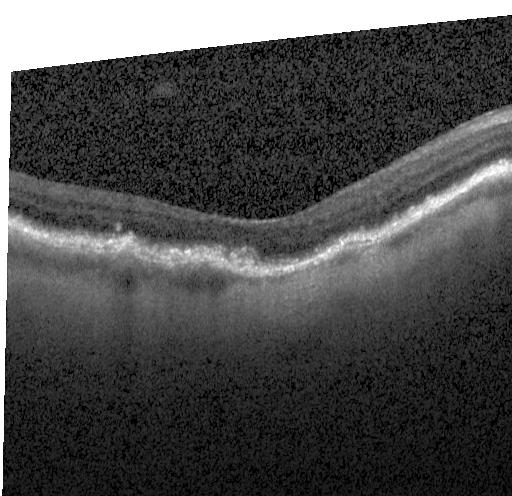
OCT B-scan — Impression: CNV.